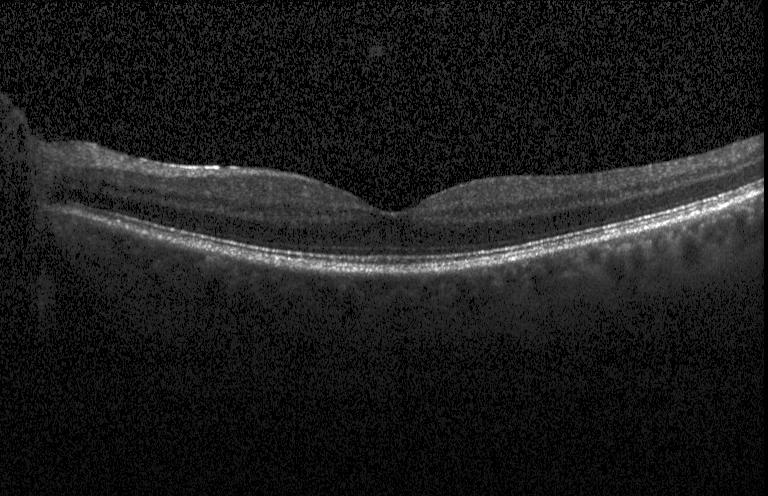
Optical coherence tomography scan
Assessment: no evidence of CNV, DME, or drusen.